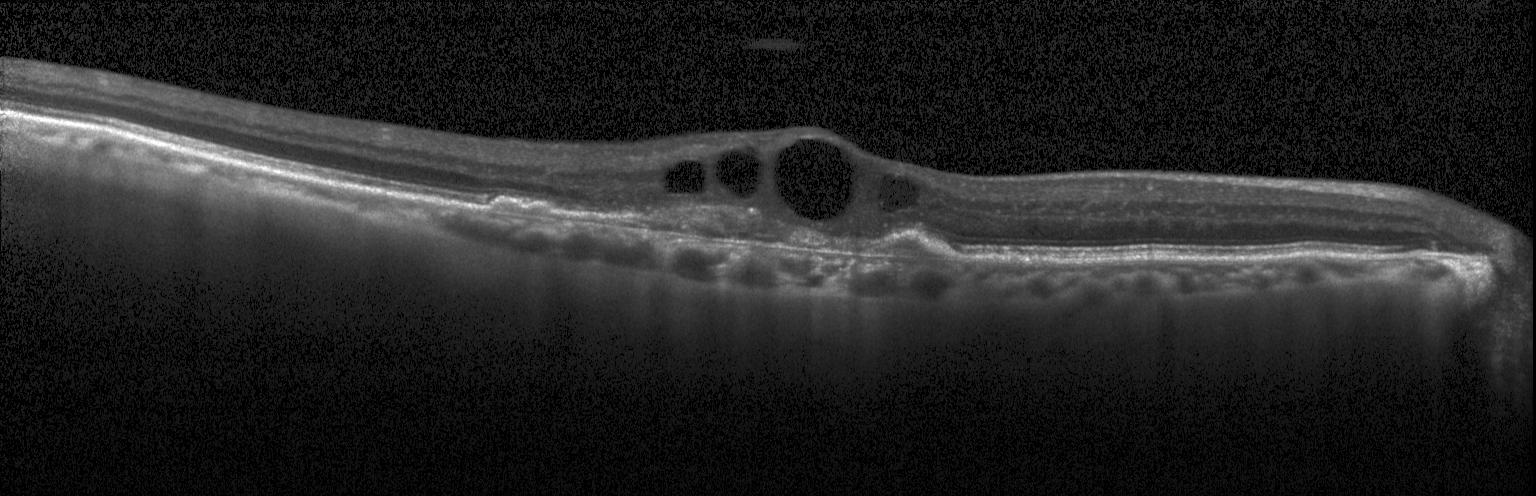

Dx: CNV.